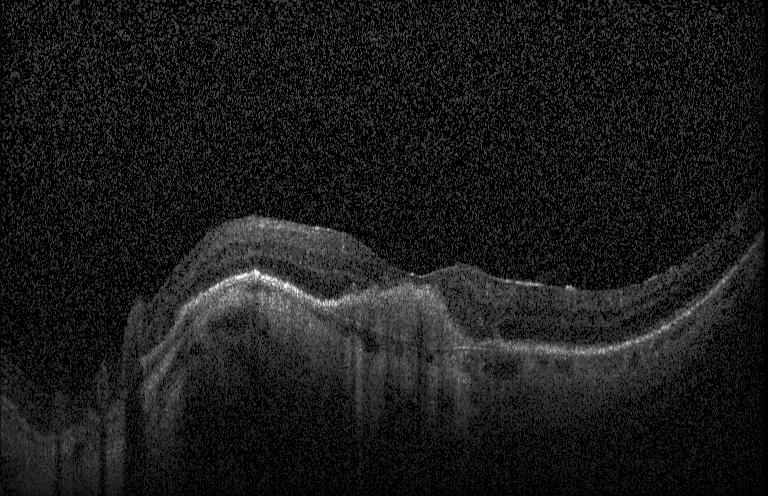 Dx: a choroidal neovascular membrane.